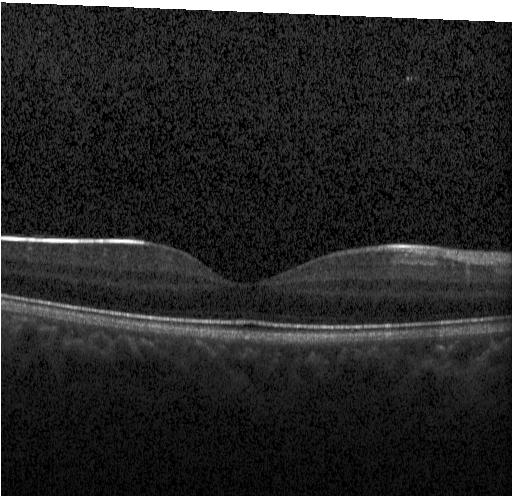
OCT line scan; acquired on a Heidelberg Spectralis; spectral-domain optical coherence tomography. The scan shows neither CNV, DME, nor drusen.